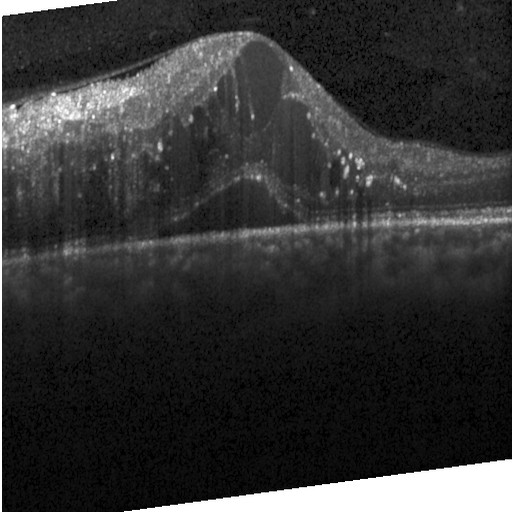

Finding: diabetic macular edema (DME).